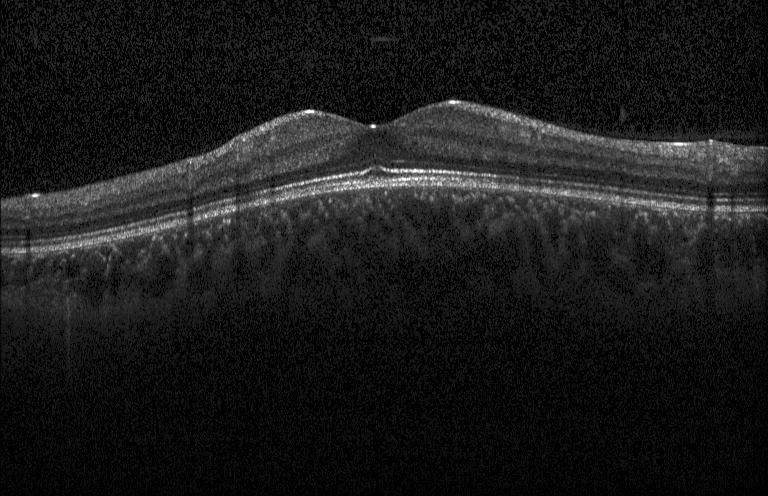
Retinal OCT B-scan, horizontal scan through the fovea, Heidelberg Spectralis, spectral-domain OCT — Finding: no choroidal neovascularization, diabetic macular edema, or drusen.